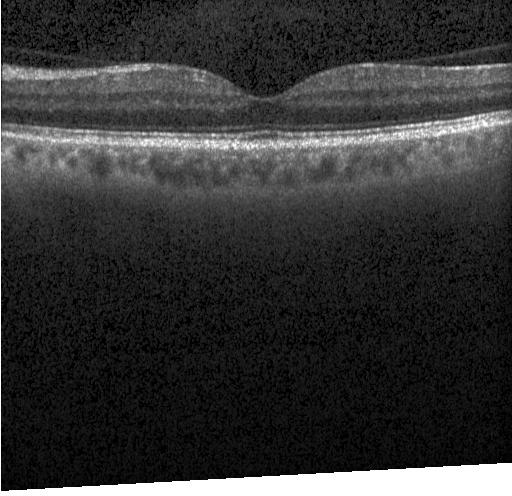 Spectral-domain OCT B-scan: no CNV, DME, or drusen.